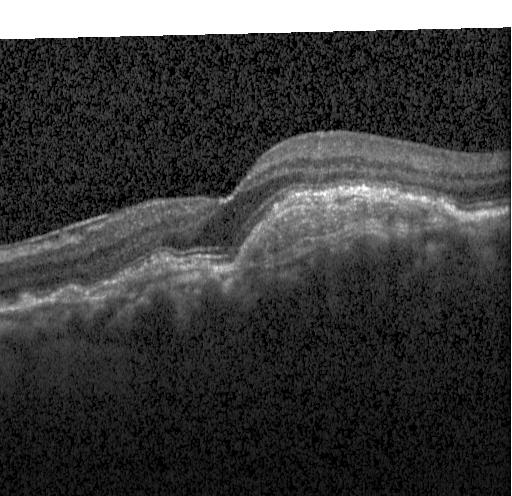
This B-scan demonstrates choroidal neovascularization.